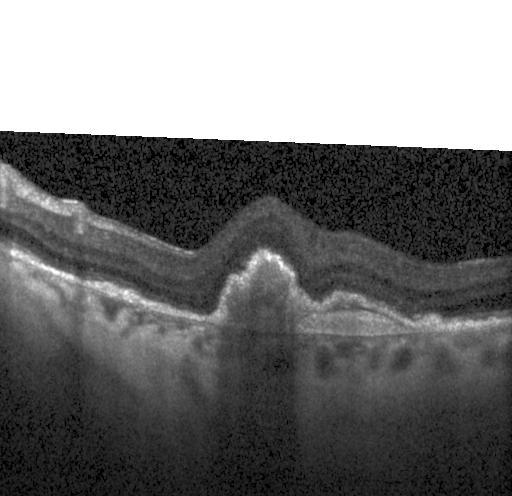

A choroidal neovascular membrane.